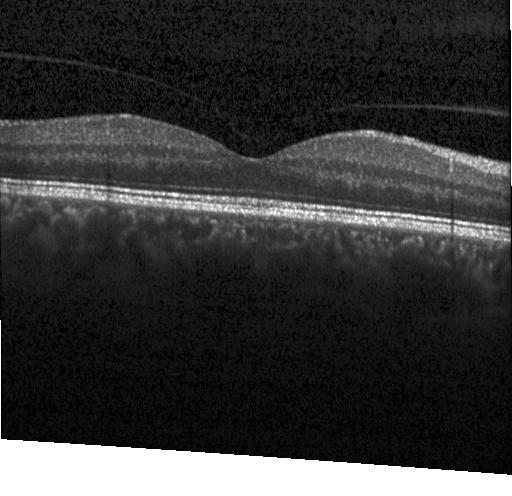 OCT line scan, SD-OCT — The scan shows no choroidal neovascularization, no diabetic macular edema, and no drusen.